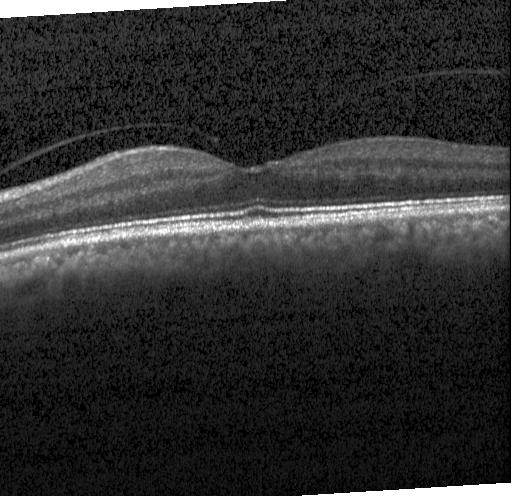
Centered on the fovea. OCT B-scan
The scan shows no choroidal neovascularization, diabetic macular edema, or drusen.